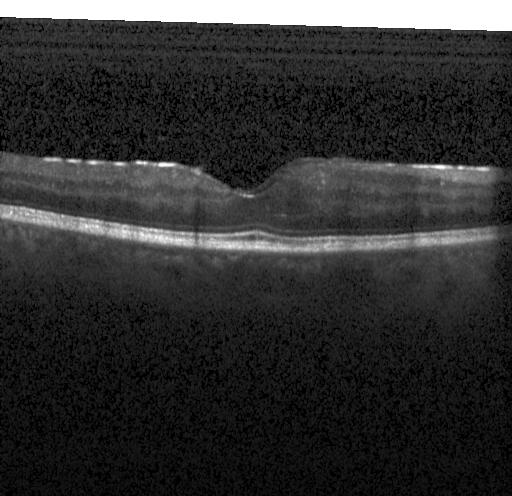 Macular OCT demonstrating neither CNV, DME, nor drusen.